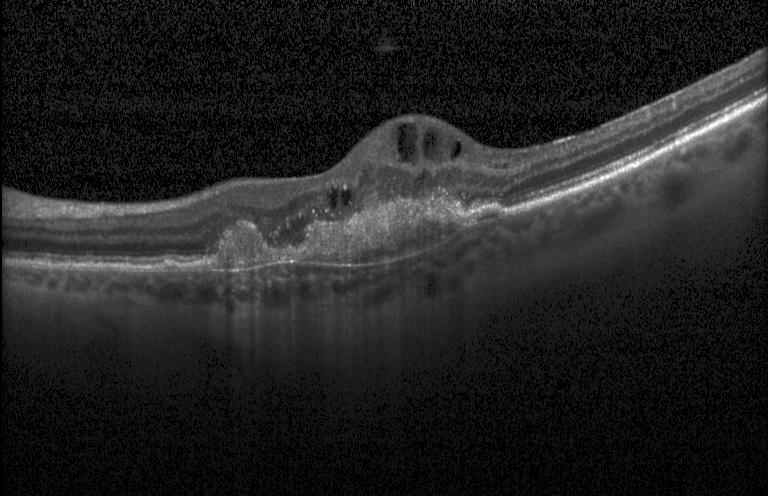

Acquired on a Heidelberg Spectralis; centered on the fovea; optical coherence tomography scan; spectral-domain OCT
Impression: choroidal neovascularization.